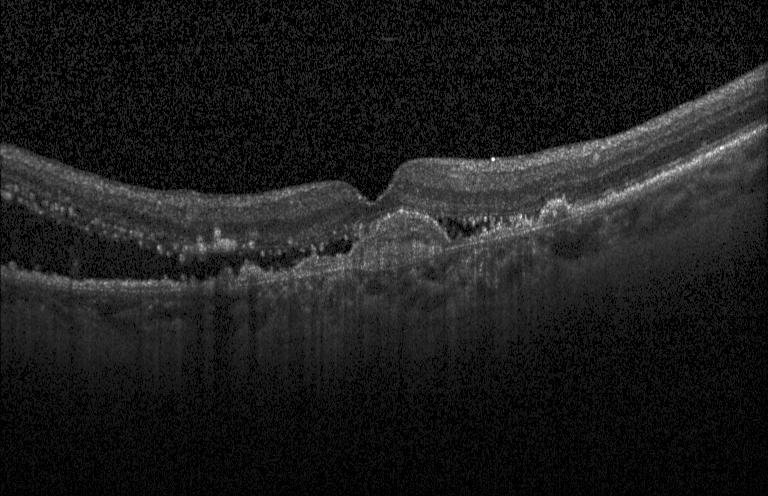
Impression: a choroidal neovascular membrane.